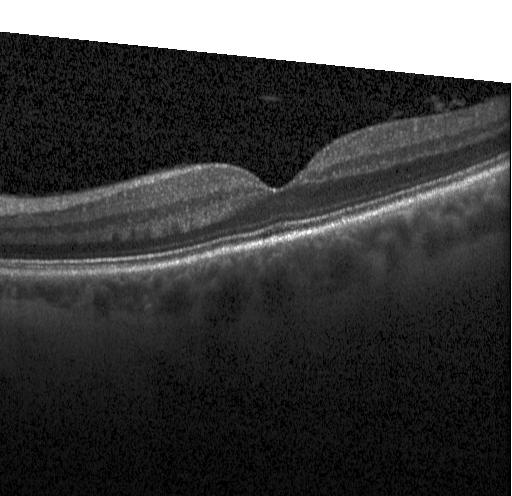
Optical coherence tomography B-scan · spectral-domain optical coherence tomography · Heidelberg Spectralis · horizontal scan through the fovea.
Diagnosis: no evidence of CNV, DME, or drusen.